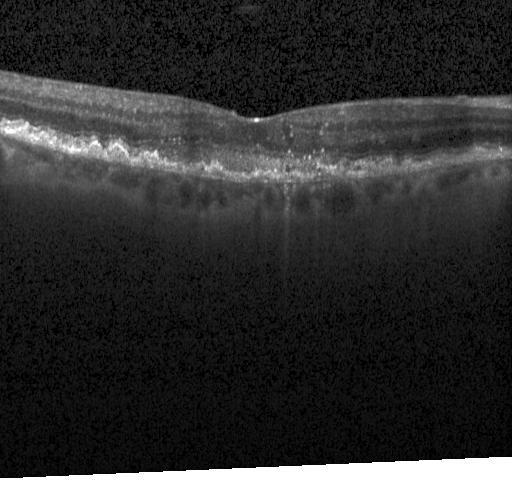

Macular scan · retinal OCT cross-section · spectral-domain OCT · Heidelberg Spectralis.
Finding: choroidal neovascularization.